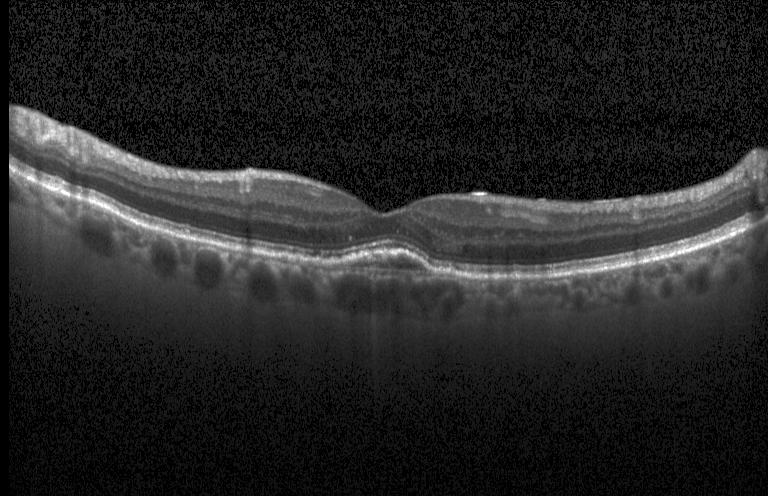

Retinal OCT B-scan.
Finding: a choroidal neovascular membrane.